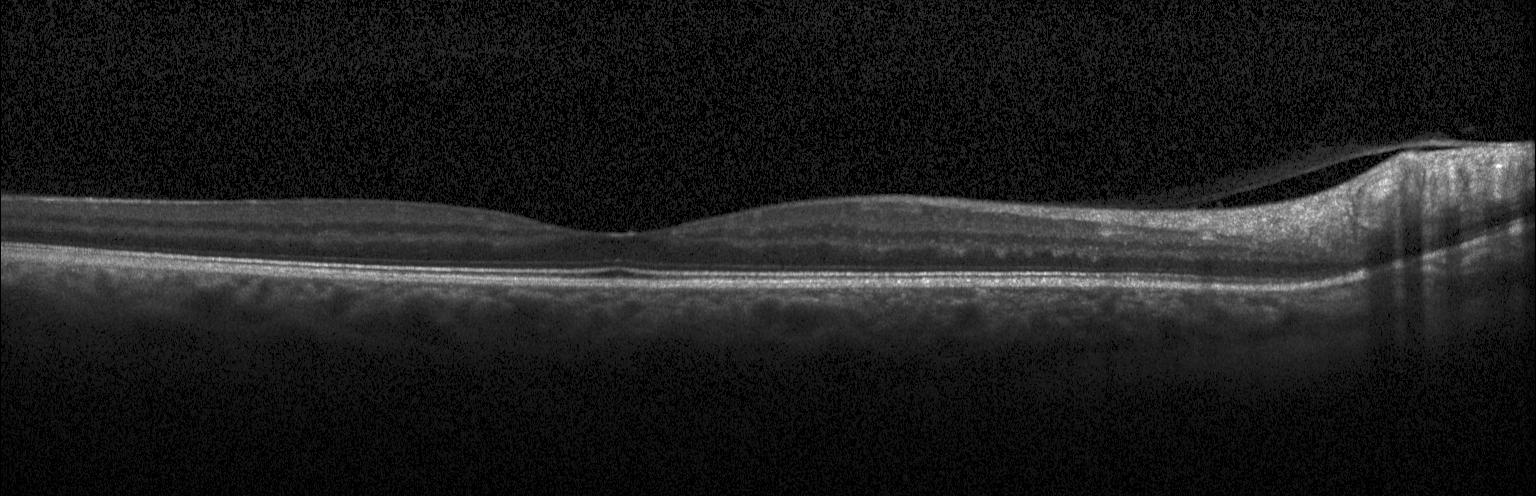 Spectral-domain OCT, acquired on a Heidelberg Spectralis, optical coherence tomography scan
This B-scan demonstrates neither CNV, DME, nor drusen.